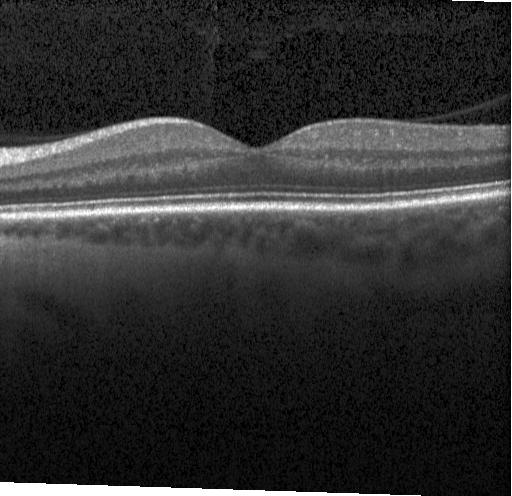 Macular scan. OCT B-scan — Diagnosis: neither choroidal neovascularization, diabetic macular edema, nor drusen.